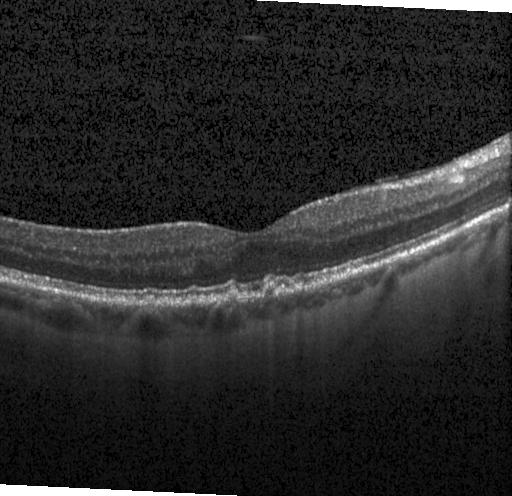 Retinal OCT cross-section, spectral-domain OCT, instrument: Heidelberg Spectralis. Finding: multiple drusen.